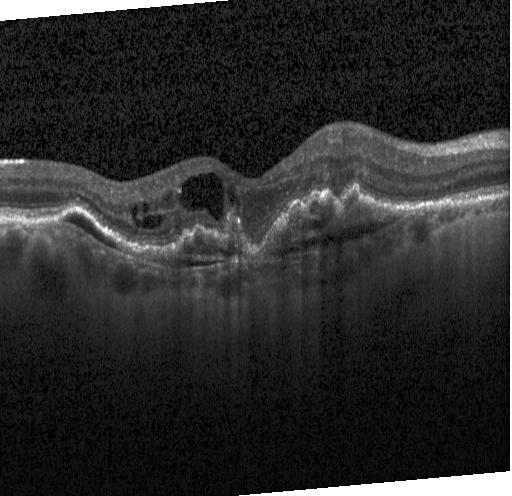 Heidelberg Spectralis OCT system, spectral-domain optical coherence tomography, retinal OCT B-scan
Macular OCT: a choroidal neovascular membrane.